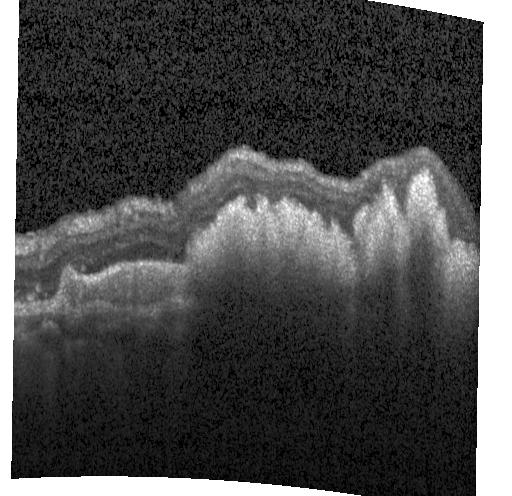

OCT finding: a choroidal neovascular membrane.